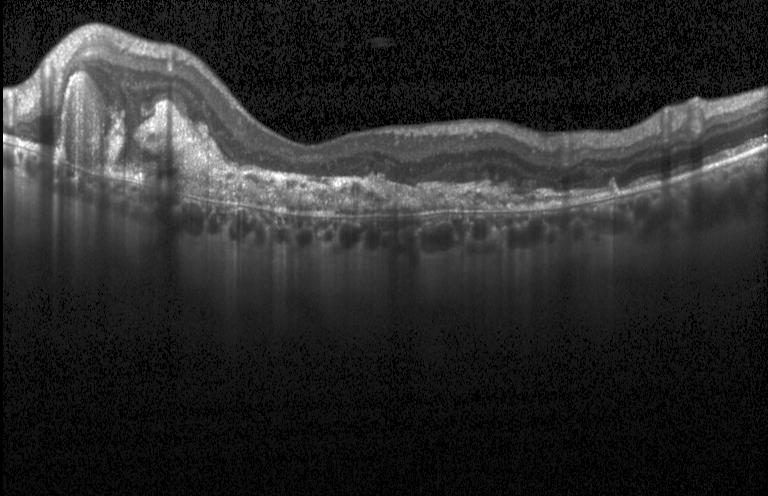 Heidelberg Spectralis, SD-OCT, retinal OCT cross-section. Assessment: a choroidal neovascular membrane.